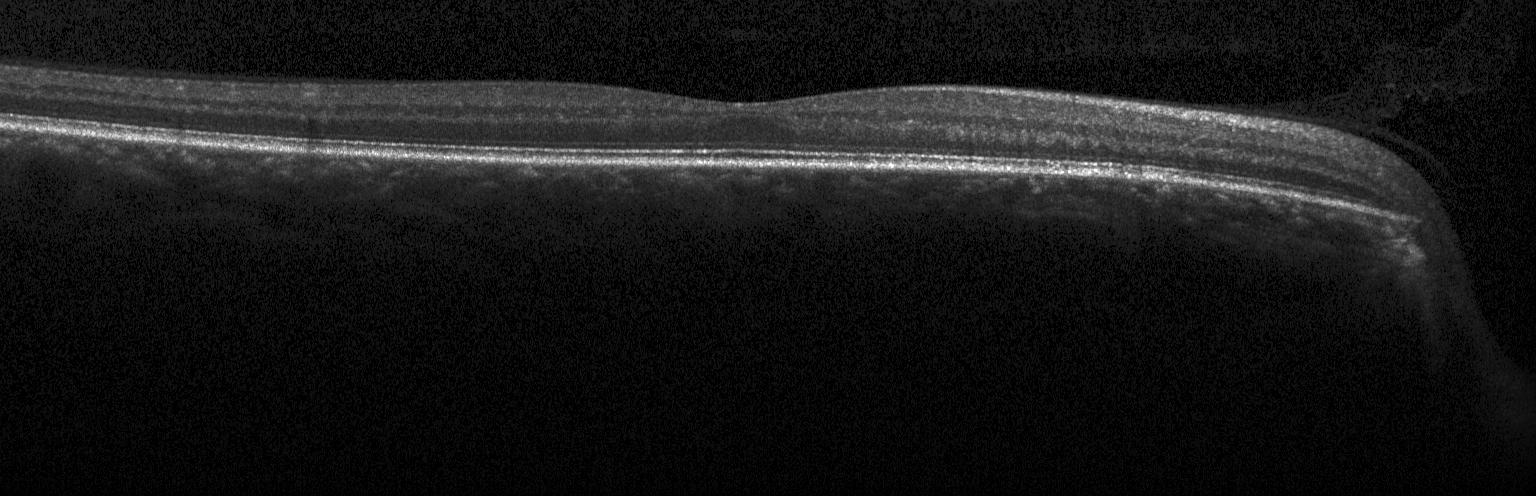 Optical coherence tomography scan, Heidelberg Spectralis
Diagnosis: no choroidal neovascularization, no diabetic macular edema, and no drusen.